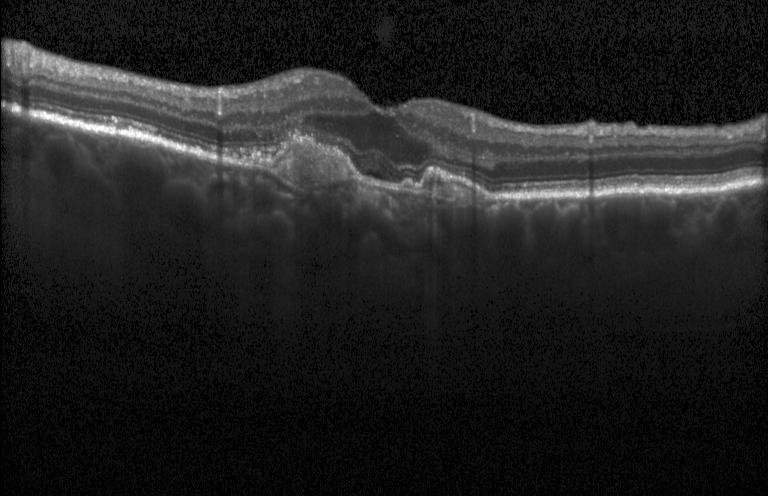

Retinal OCT B-scan
The scan shows CNV.